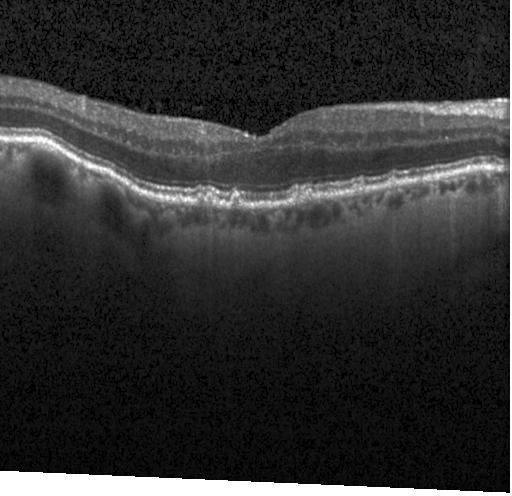

Sub-RPE drusenoid deposits.